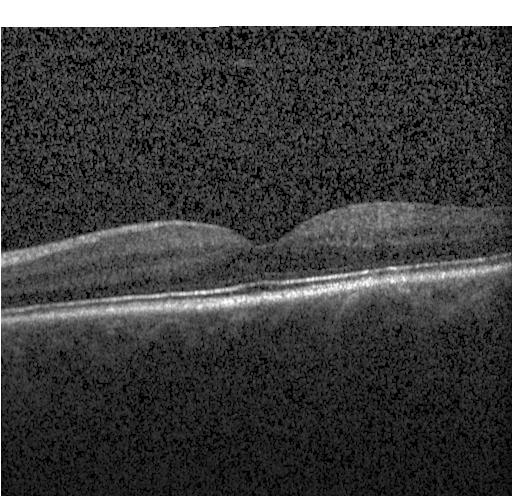
Heidelberg Spectralis OCT system, OCT line scan, fovea-centered — The scan shows no CNV, no DME, and no drusen.